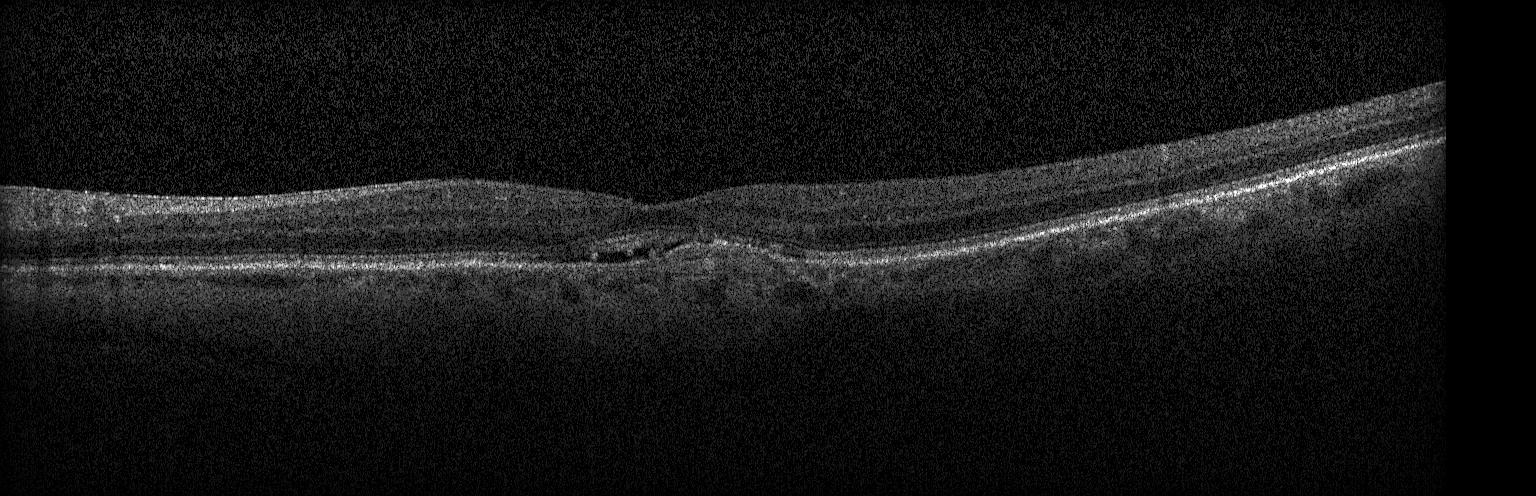
Macular OCT demonstrating a choroidal neovascular membrane.